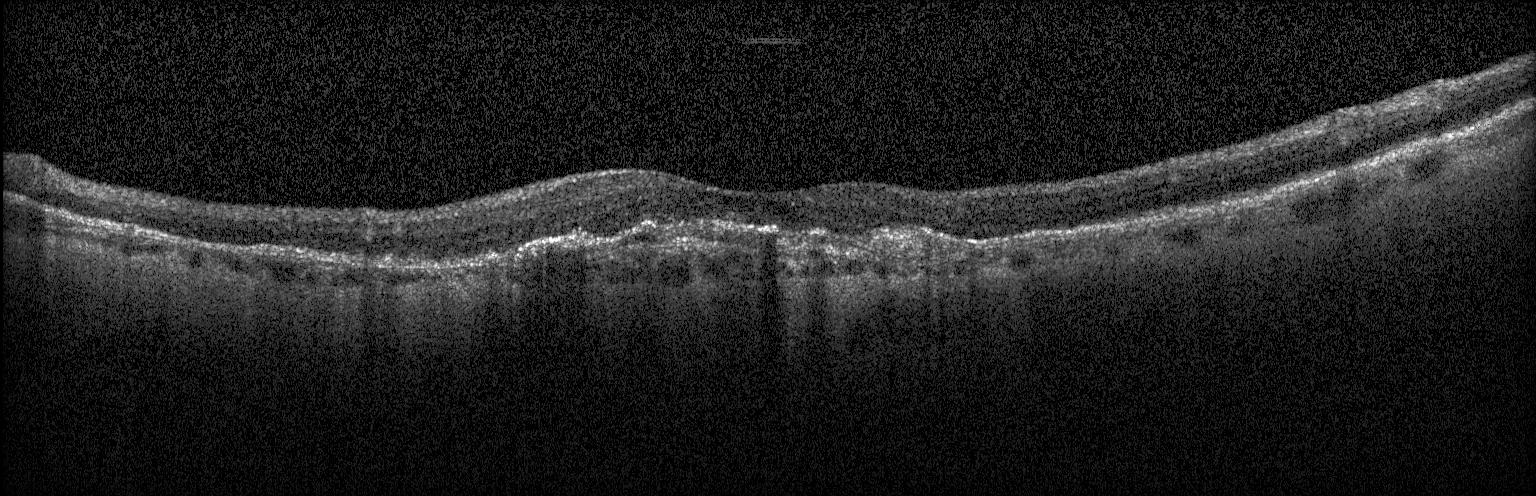 Spectral-domain OCT. Instrument: Heidelberg Spectralis. OCT B-scan. Fovea-centered. OCT finding: a choroidal neovascular membrane.